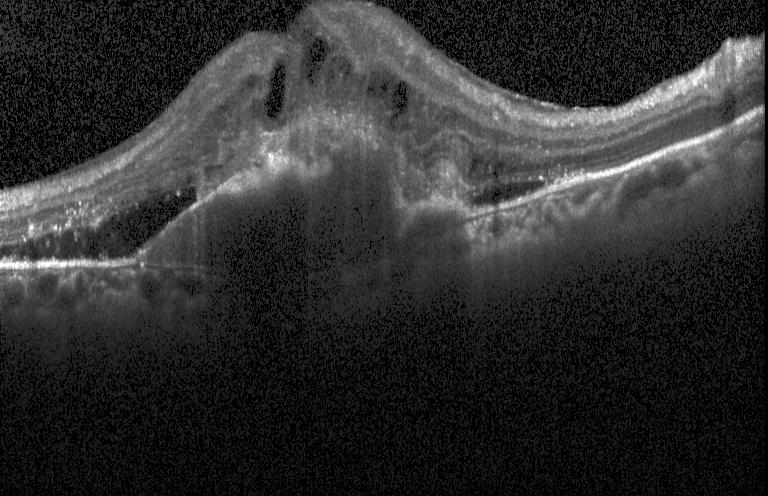

OCT line scan · Heidelberg Spectralis. Impression: choroidal neovascularization (CNV).